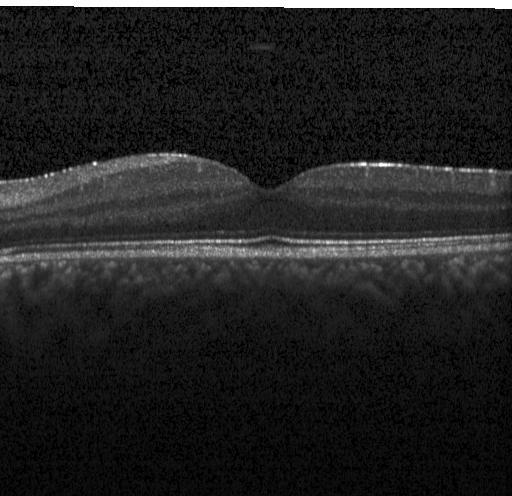 No evidence of choroidal neovascularization, diabetic macular edema, or drusen.